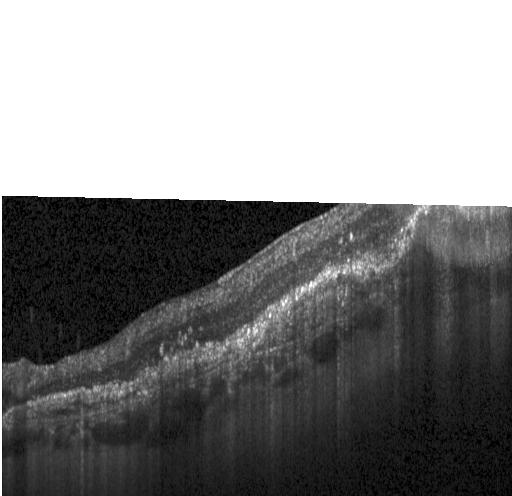

Optical coherence tomography scan. Heidelberg Spectralis — Finding: choroidal neovascularization (CNV).